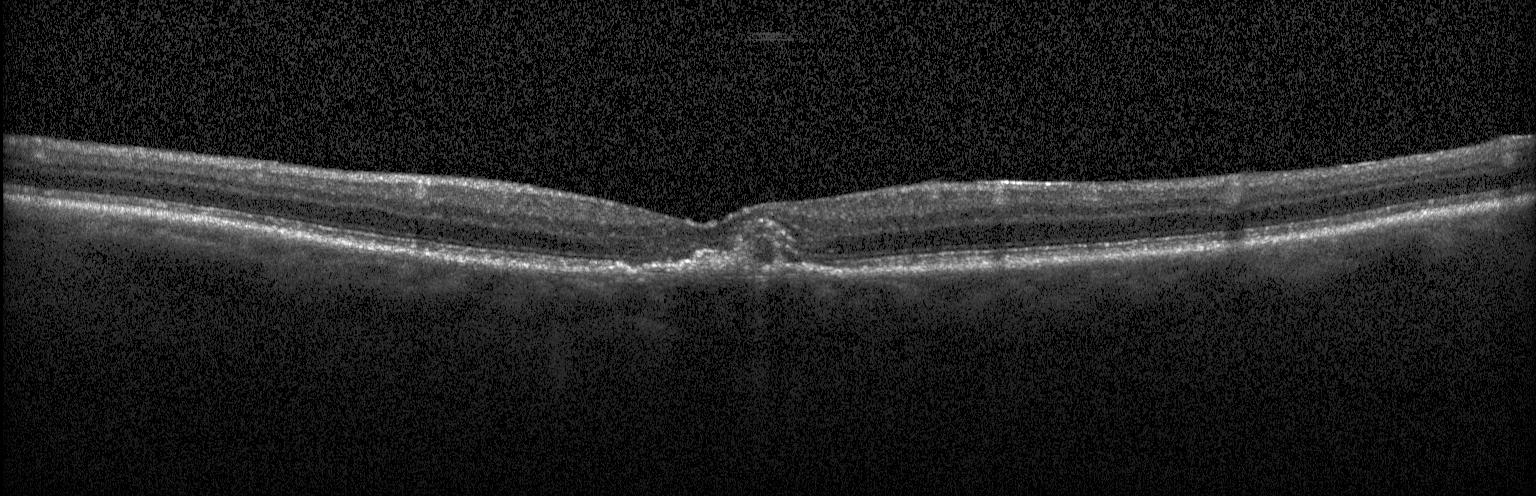
OCT line scan — Diagnosis: CNV.